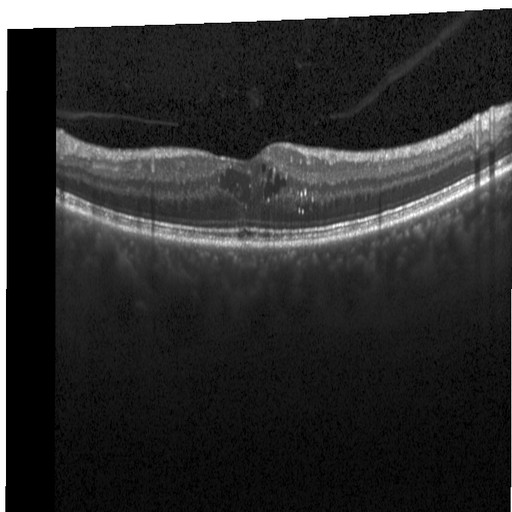 OCT B-scan · SD-OCT · acquired on a Heidelberg Spectralis — Assessment: diabetic macular edema (DME).